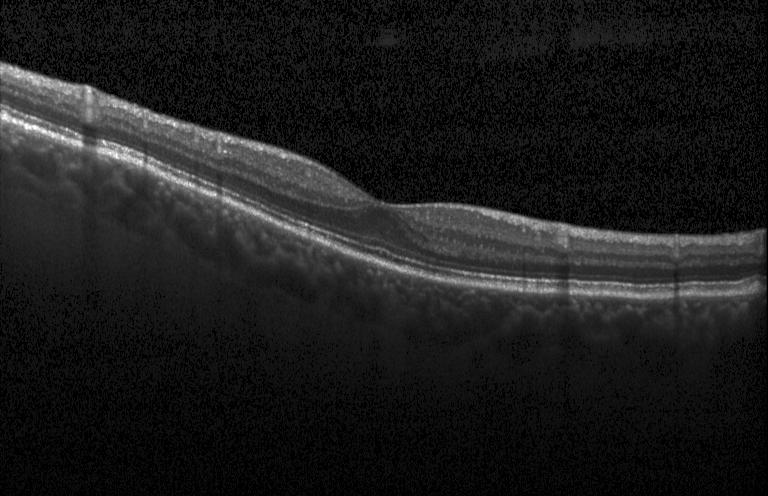

Macular scan · optical coherence tomography B-scan · instrument: Heidelberg Spectralis · spectral-domain OCT. This B-scan demonstrates no choroidal neovascularization, no diabetic macular edema, and no drusen.